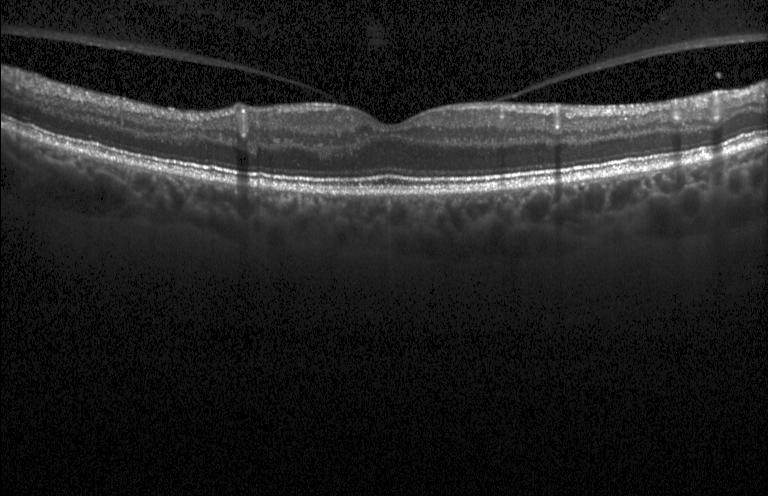
Through the macula; retinal OCT B-scan. Finding: no CNV, DME, or drusen.